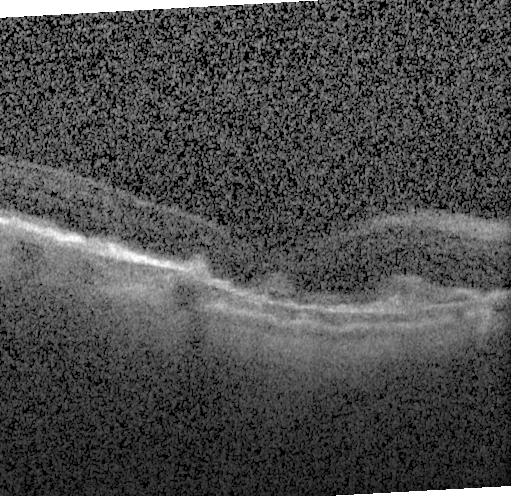
OCT line scan. Spectral-domain OCT. Centered on the fovea. This B-scan demonstrates a choroidal neovascular membrane.